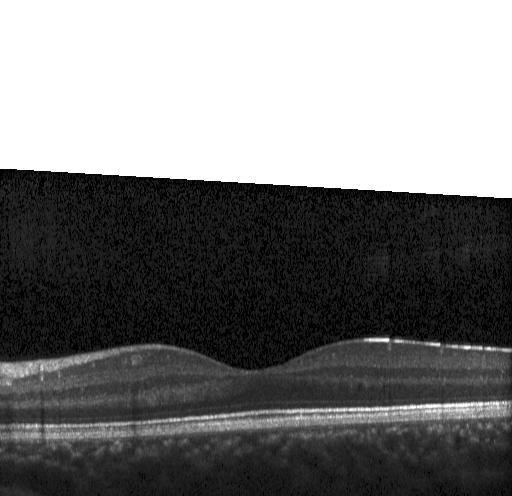

Diagnosis: no evidence of choroidal neovascularization, diabetic macular edema, or drusen.